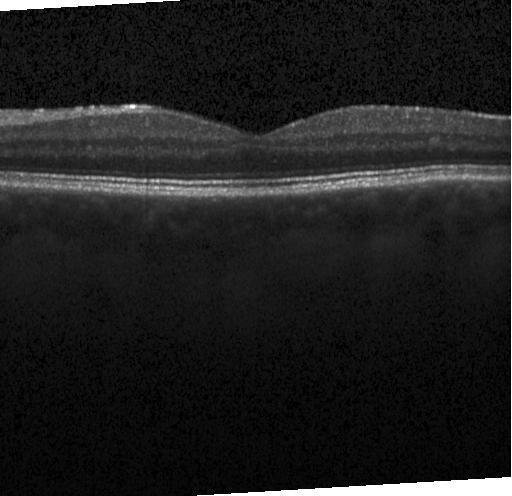 Diagnosis: no choroidal neovascularization, no diabetic macular edema, and no drusen.